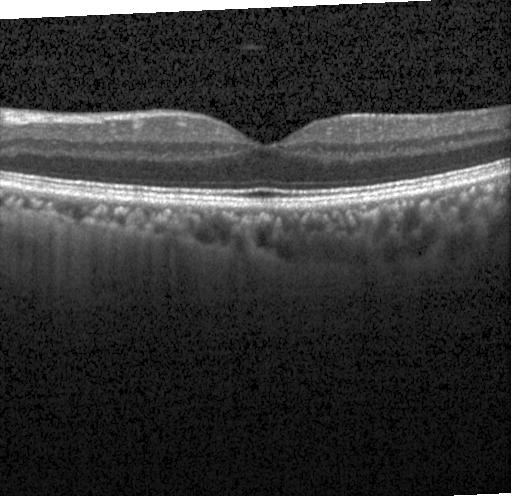

OCT B-scan showing no evidence of choroidal neovascularization, diabetic macular edema, or drusen.